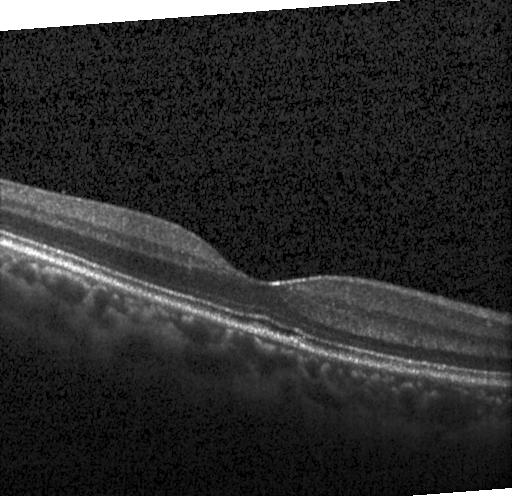
Retinal OCT cross-section.
Diagnosis: no choroidal neovascularization, diabetic macular edema, or drusen.